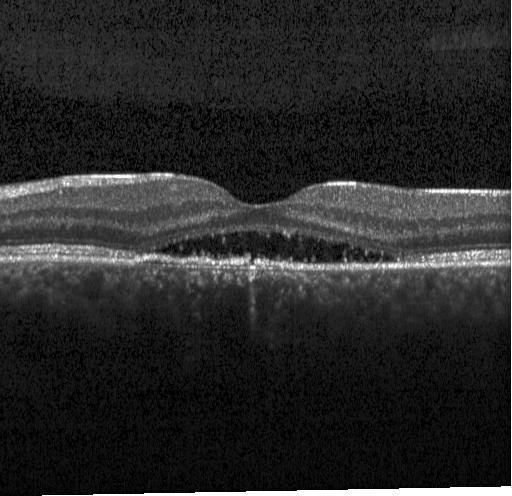

Spectral-domain OCT. Optical coherence tomography B-scan — Dx: choroidal neovascularization.